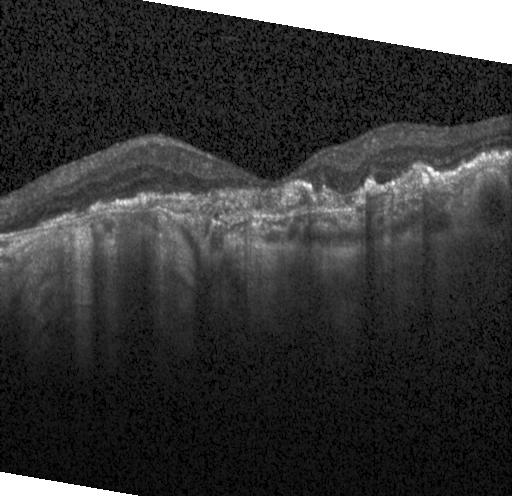 Macular scan. Retinal OCT B-scan. Spectral-domain OCT
Dx: CNV.